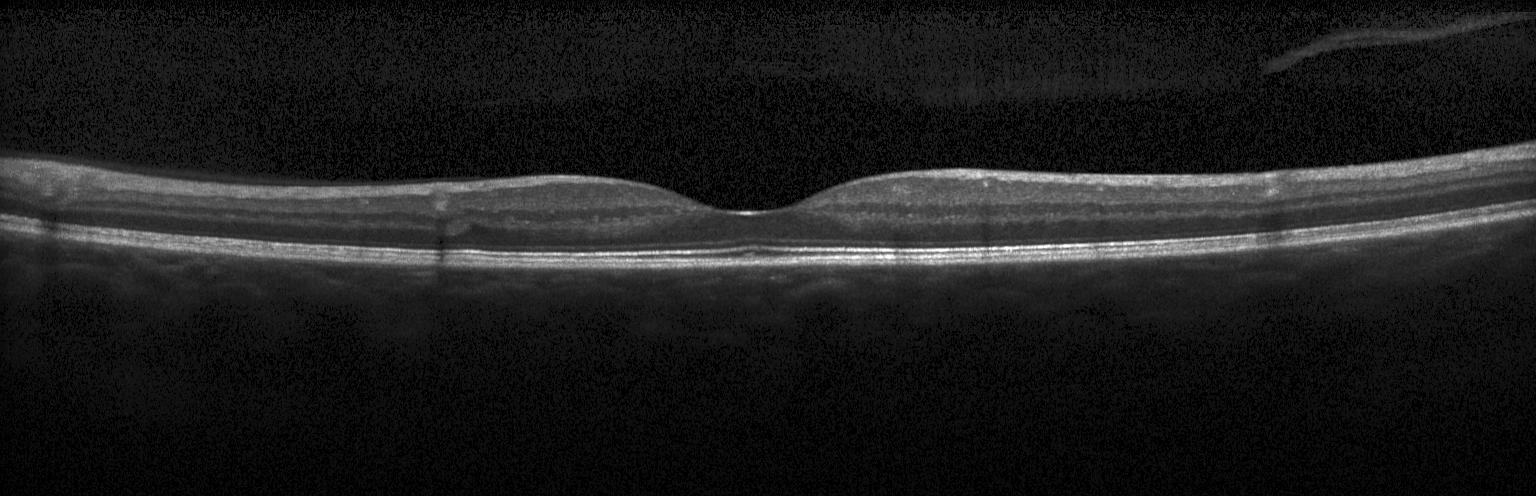

Dx: neither choroidal neovascularization, diabetic macular edema, nor drusen.